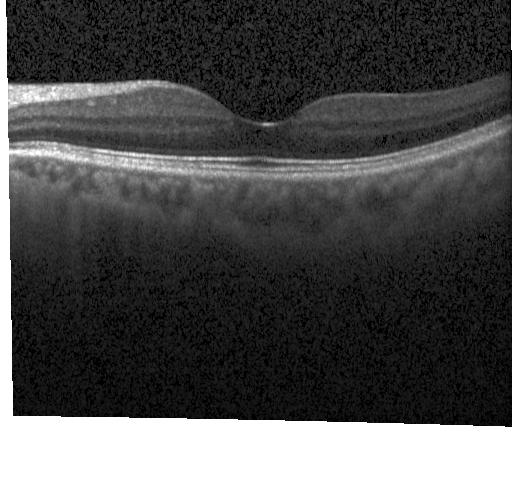 Impression: no choroidal neovascularization, no diabetic macular edema, and no drusen.